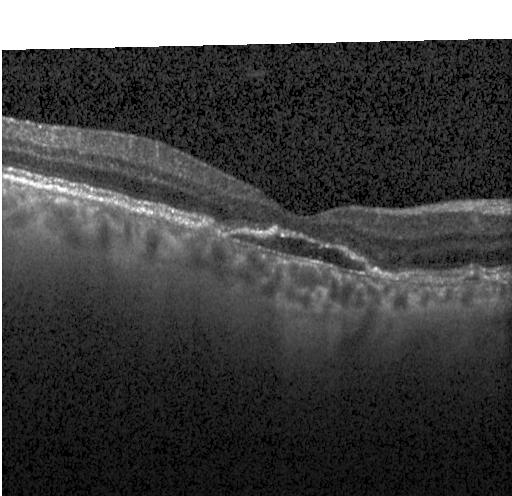

OCT B-scan showing CNV.